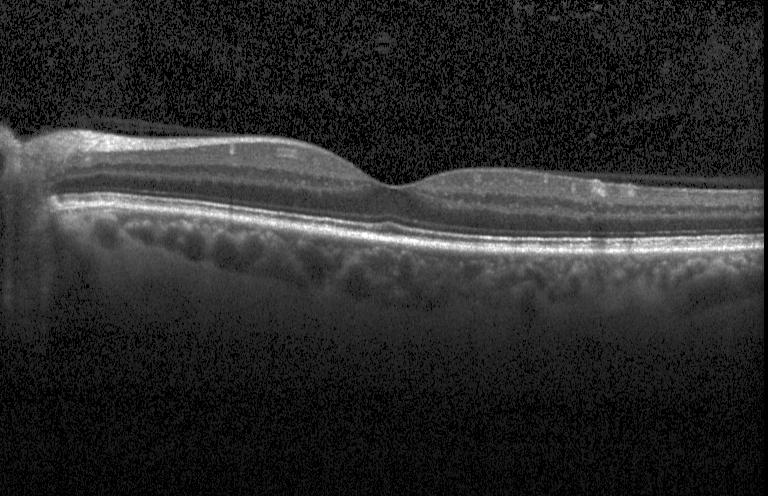
Spectral-domain OCT B-scan: no evidence of CNV, DME, or drusen.